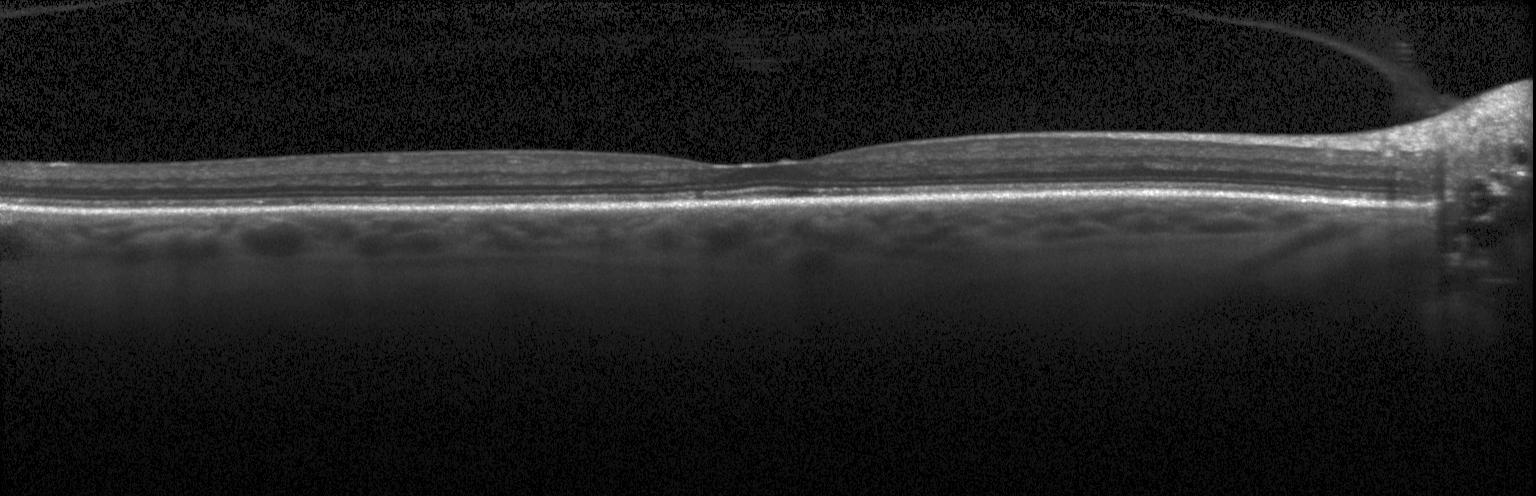
Impression: no choroidal neovascularization, diabetic macular edema, or drusen.